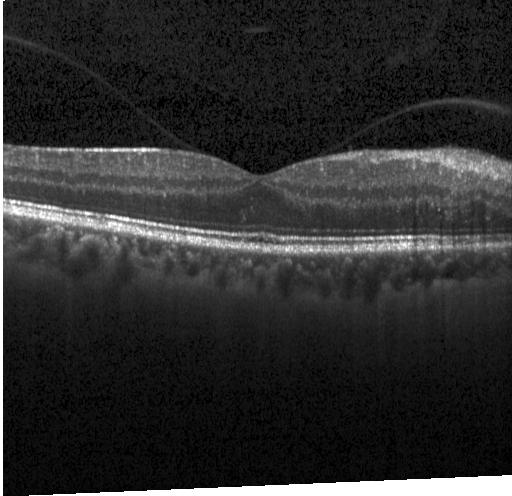 Retinal OCT cross-section.
The scan shows neither choroidal neovascularization, diabetic macular edema, nor drusen.